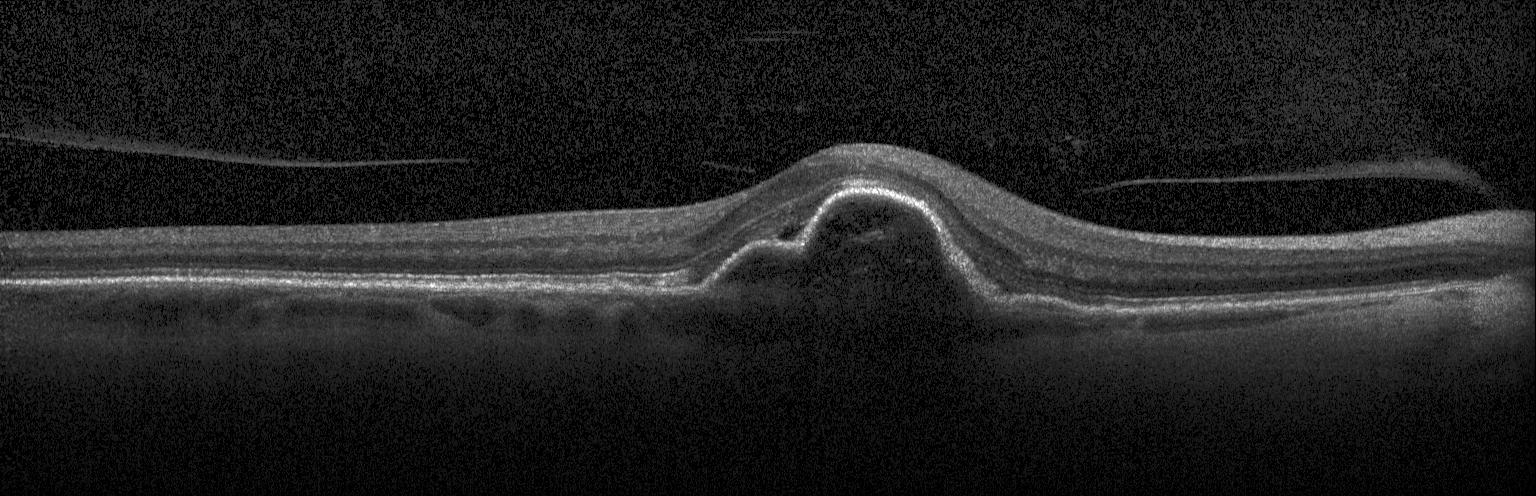

Heidelberg Spectralis, SD-OCT, OCT line scan. Macular OCT: a choroidal neovascular membrane.